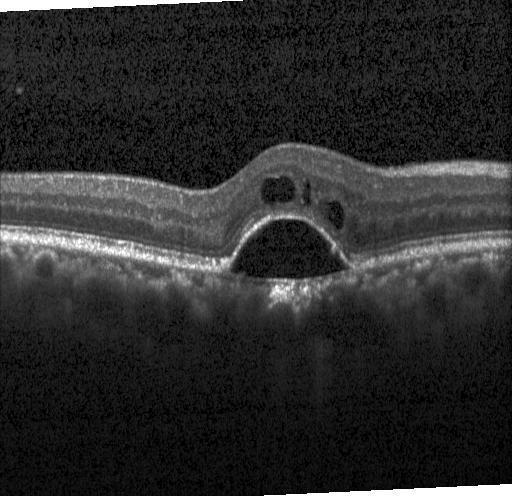 Spectral-domain OCT B-scan: a choroidal neovascular membrane.